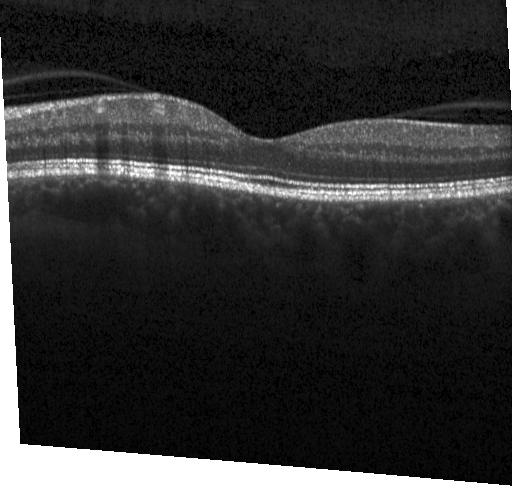

OCT B-scan showing no choroidal neovascularization, no diabetic macular edema, and no drusen.